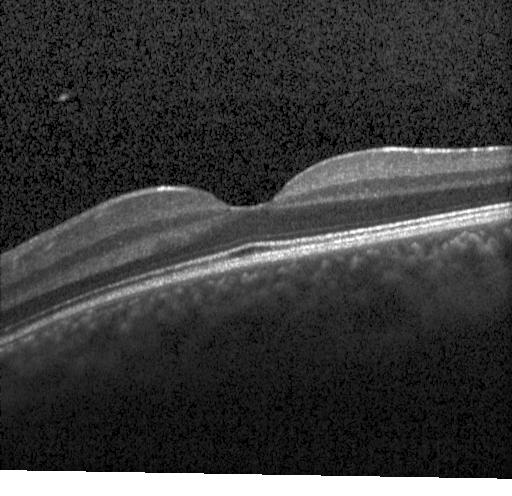
Retinal OCT B-scan. Fovea-centered — Dx: neither choroidal neovascularization, diabetic macular edema, nor drusen.